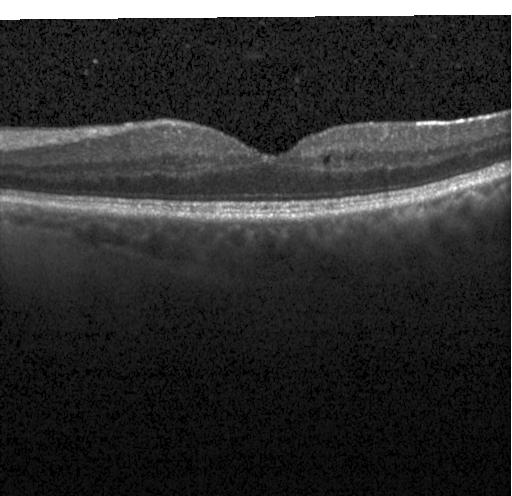

Heidelberg Spectralis OCT system, OCT line scan, spectral-domain optical coherence tomography, horizontal scan through the fovea — OCT finding: diabetic macular edema.